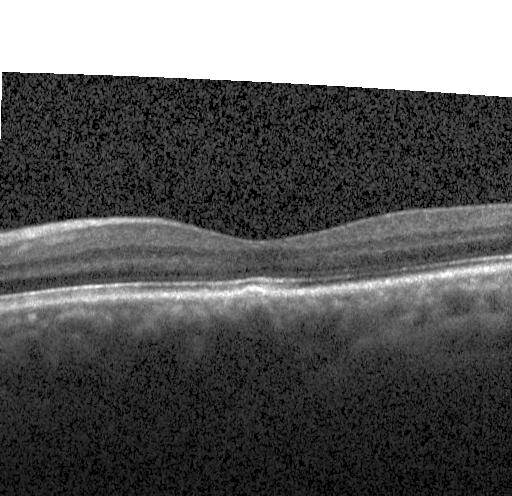 The scan shows drusen.